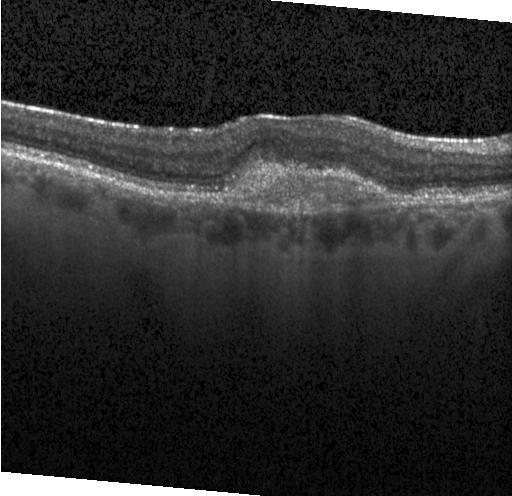 Finding: choroidal neovascularization (CNV).